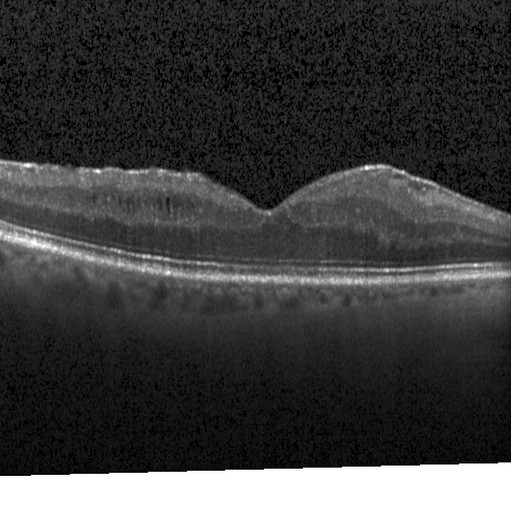 SD-OCT. Retinal OCT cross-section
Impression: diabetic macular edema (DME).